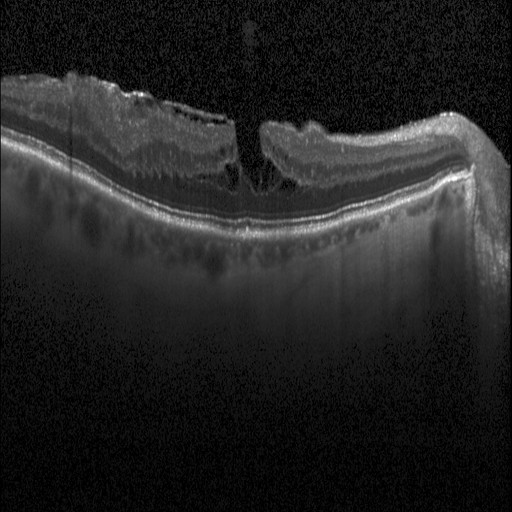

OCT scan showing diabetic macular edema (DME).